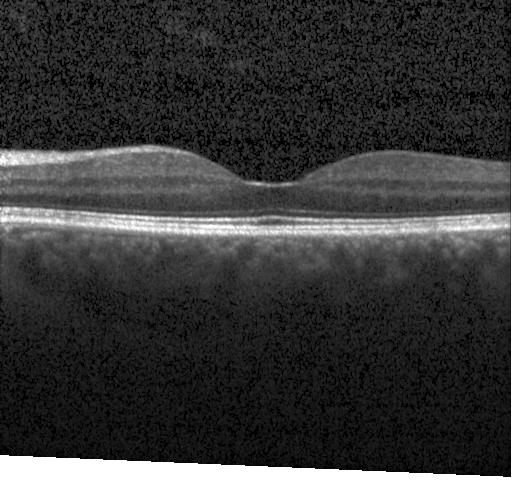

The scan shows no evidence of choroidal neovascularization, diabetic macular edema, or drusen.